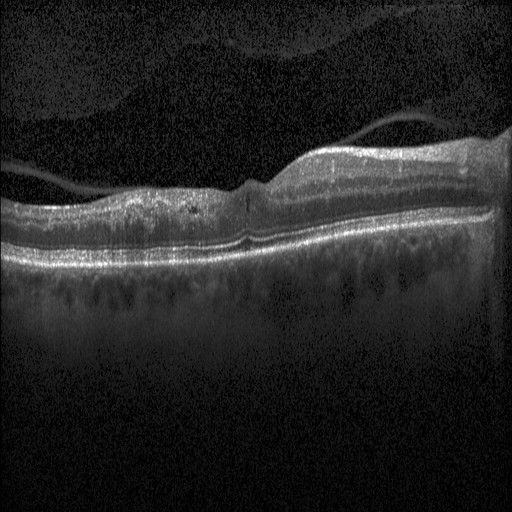 Optical coherence tomography B-scan · SD-OCT
Diagnosis: diabetic macular edema (DME).